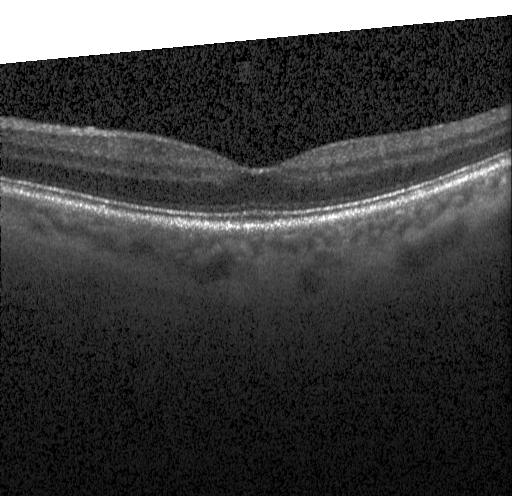
SD-OCT · optical coherence tomography B-scan · acquired on a Heidelberg Spectralis · macular scan.
The scan shows no evidence of choroidal neovascularization, diabetic macular edema, or drusen.